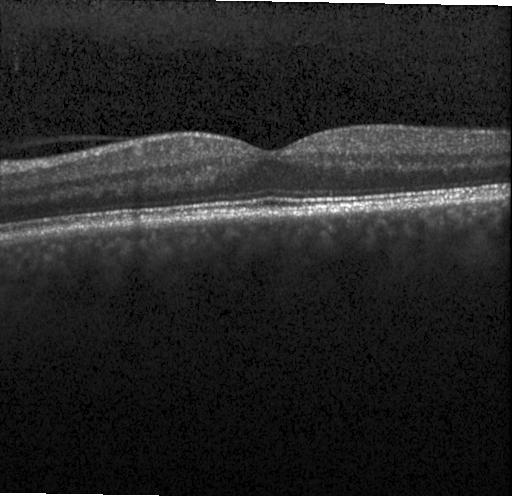
Instrument: Heidelberg Spectralis; optical coherence tomography scan
No choroidal neovascularization, no diabetic macular edema, and no drusen.